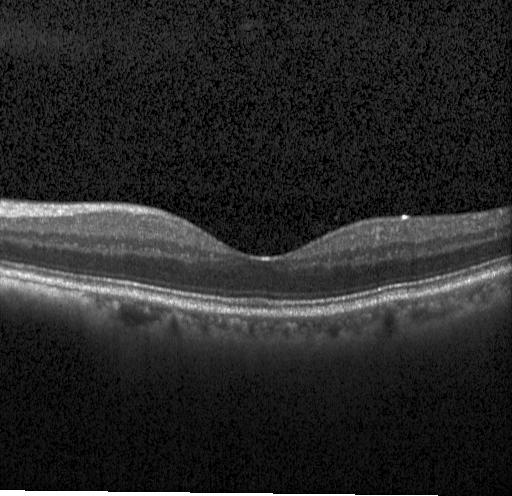

OCT B-scan
Assessment: neither CNV, DME, nor drusen.